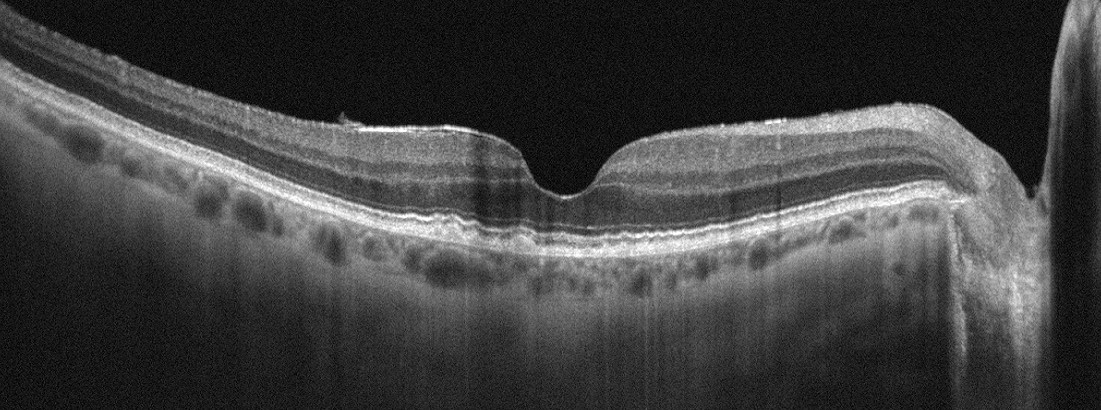
OCT line scan · through the macula · Optovue Avanti RTVue XR. OCT finding: age-related macular degeneration.